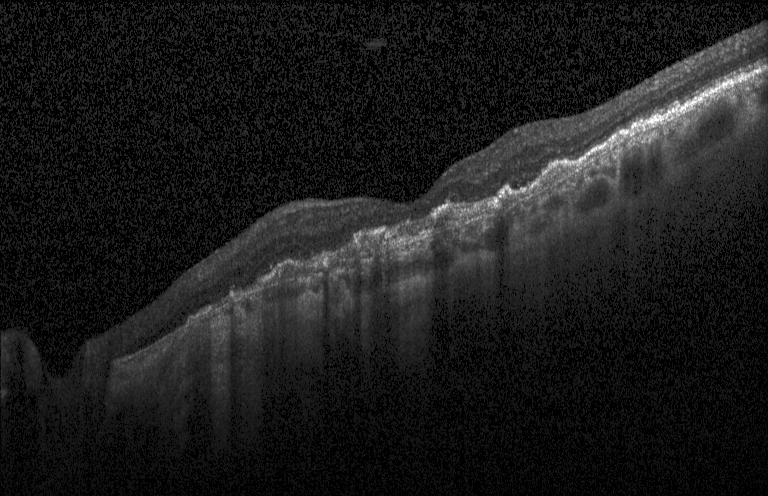

Macular OCT demonstrating a choroidal neovascular membrane.